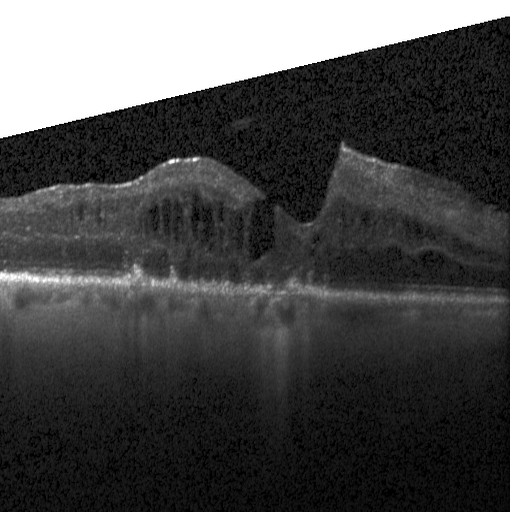

Dx: diabetic macular edema.